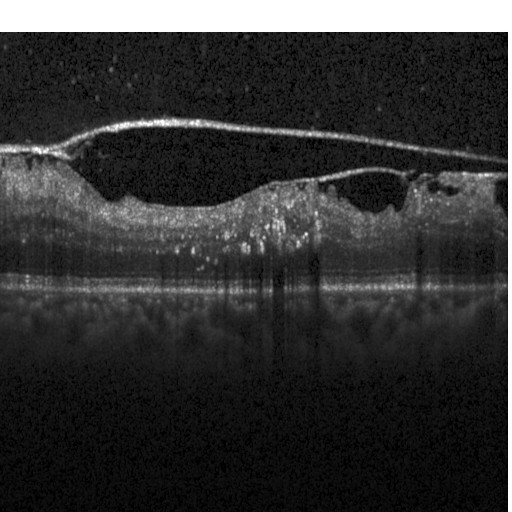

OCT B-scan
This B-scan demonstrates diabetic macular edema (DME).